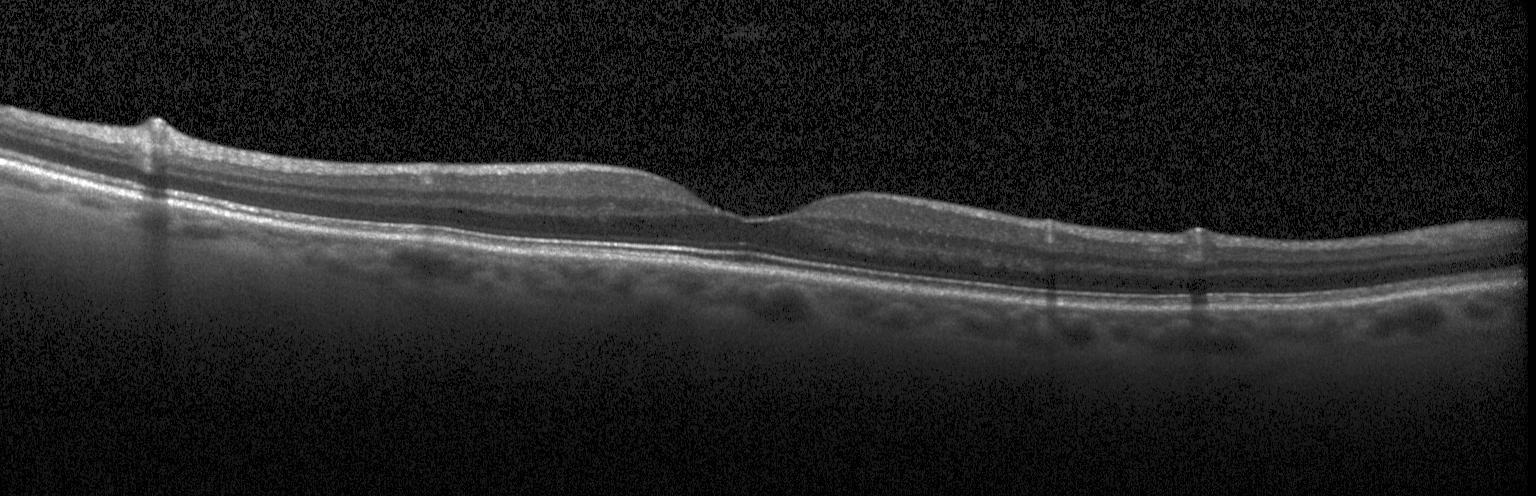 Impression: no evidence of choroidal neovascularization, diabetic macular edema, or drusen.